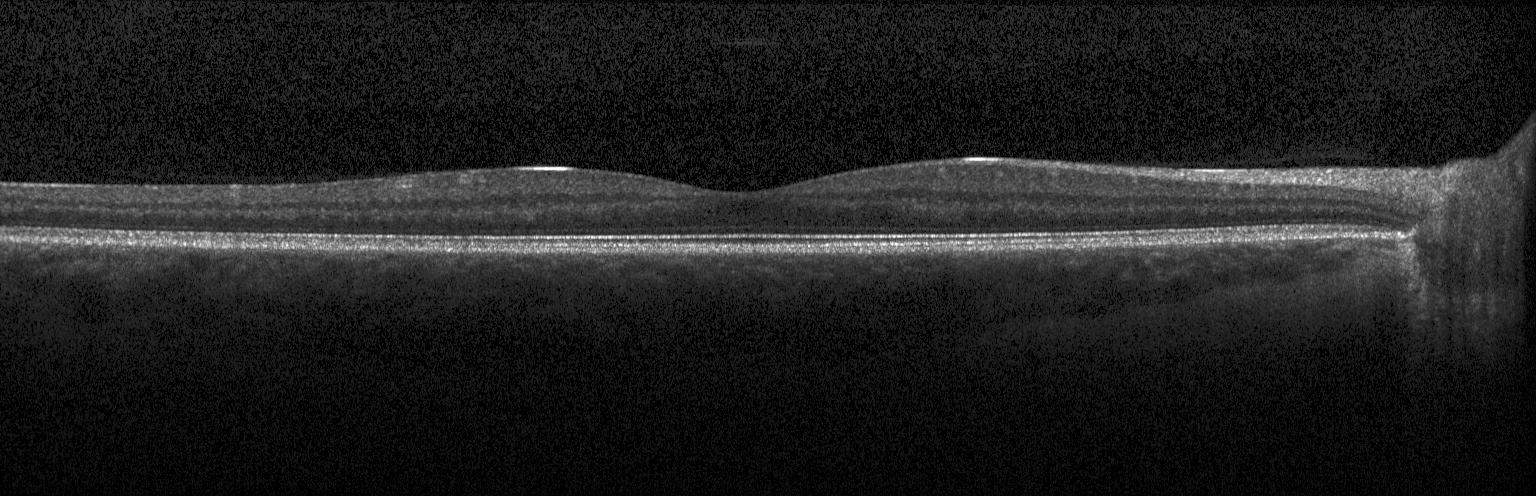 Neither choroidal neovascularization, diabetic macular edema, nor drusen.